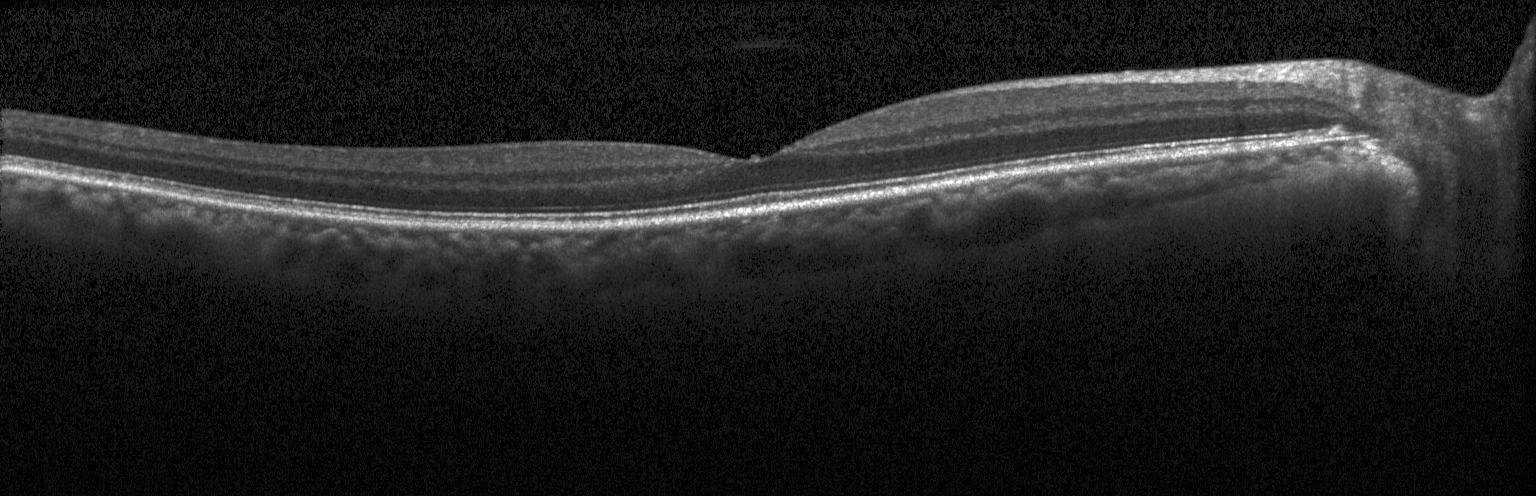 Impression: no choroidal neovascularization, no diabetic macular edema, and no drusen.